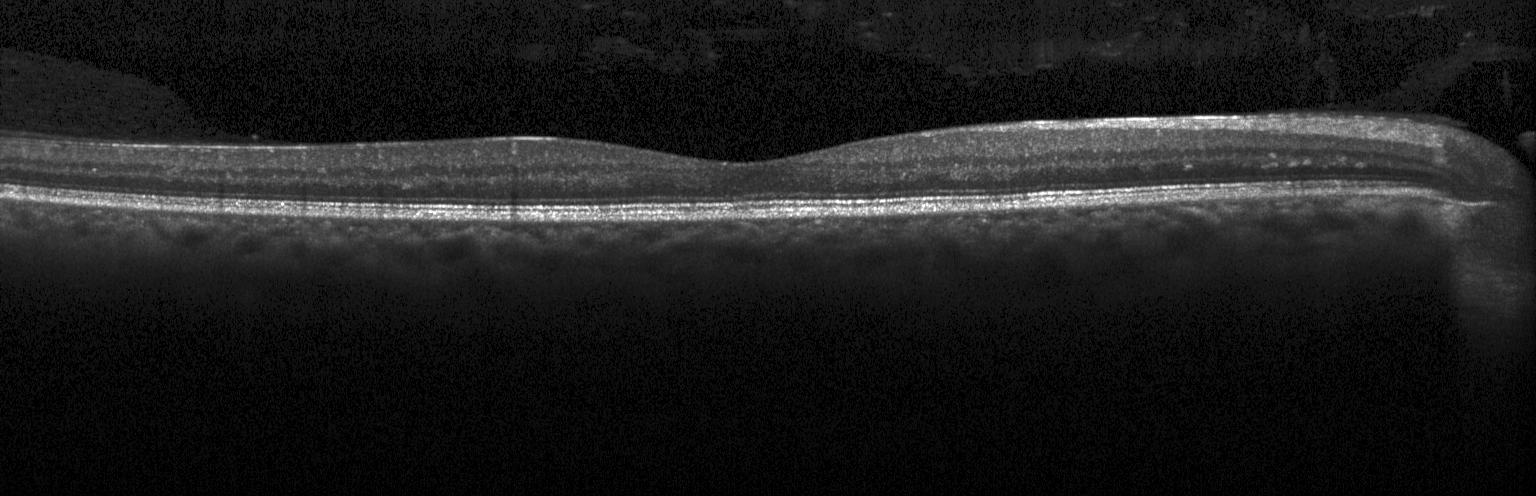

Impression: neither choroidal neovascularization, diabetic macular edema, nor drusen.